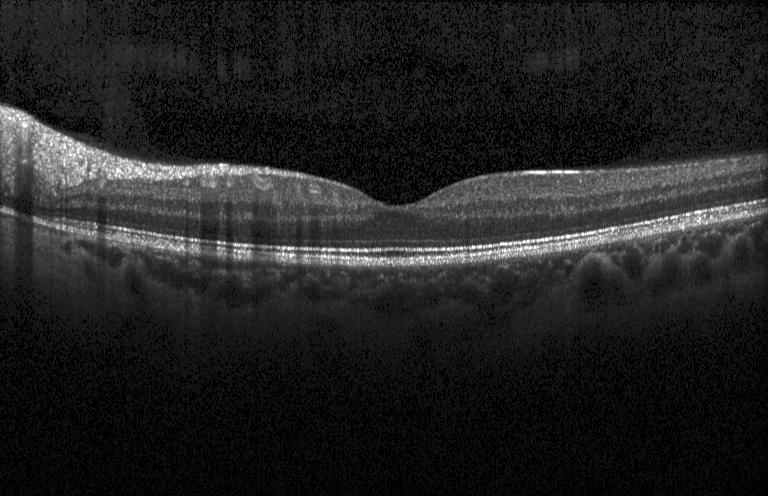 SD-OCT, through the macula, retinal OCT cross-section
Finding: no choroidal neovascularization, diabetic macular edema, or drusen.